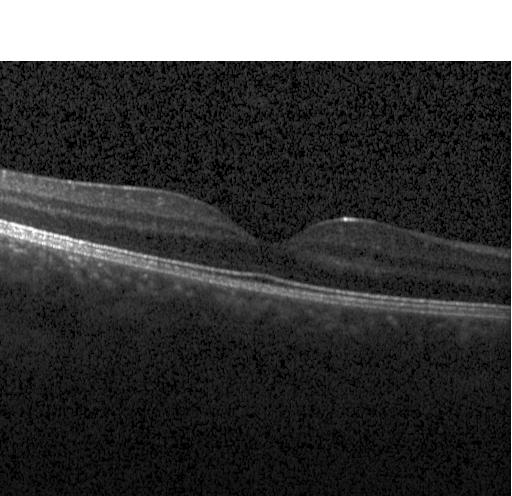 Heidelberg Spectralis OCT system; OCT B-scan
Finding: no CNV, DME, or drusen.